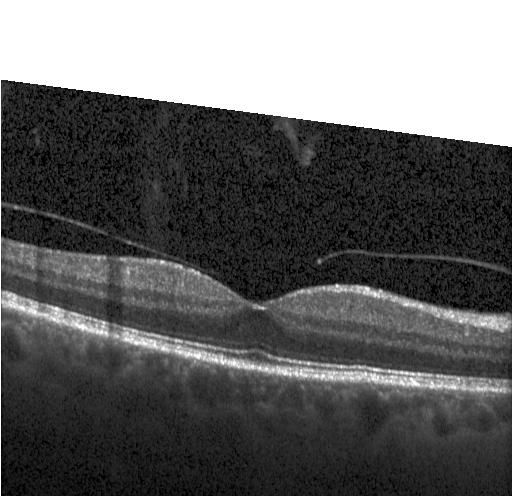 Macular OCT: no choroidal neovascularization, diabetic macular edema, or drusen.